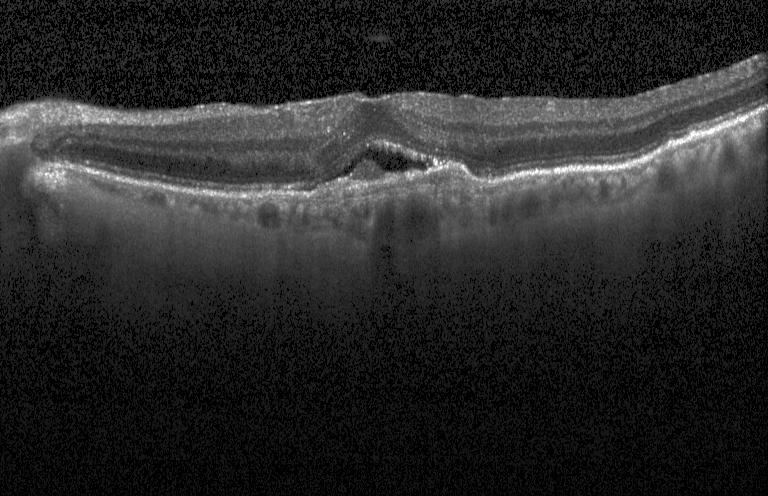

Dx: a choroidal neovascular membrane.